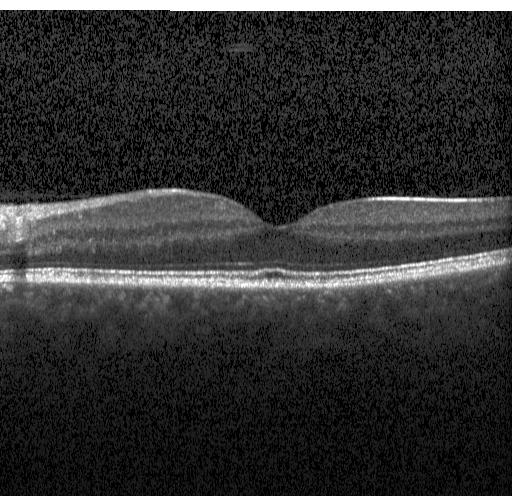
Spectral-domain OCT B-scan: no choroidal neovascularization, no diabetic macular edema, and no drusen.